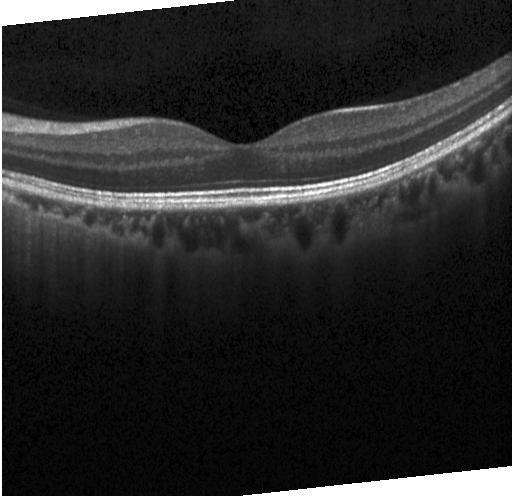

Spectral-domain optical coherence tomography; instrument: Heidelberg Spectralis; OCT line scan; through the macula. This B-scan demonstrates no choroidal neovascularization, no diabetic macular edema, and no drusen.